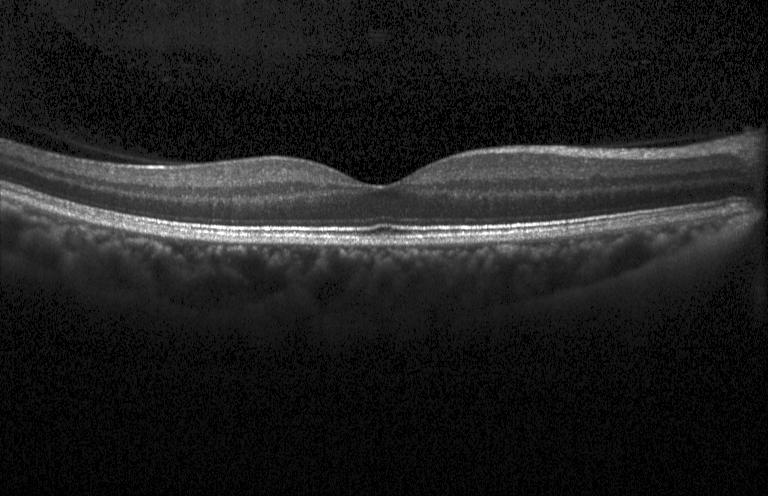
Diagnosis: no choroidal neovascularization, no diabetic macular edema, and no drusen.